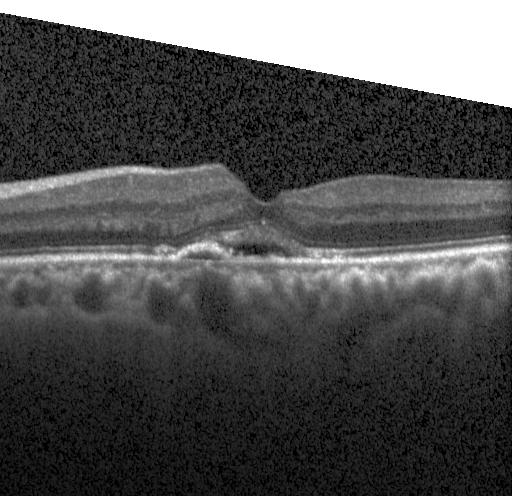
Retinal OCT B-scan; centered on the fovea; SD-OCT; instrument: Heidelberg Spectralis
This B-scan demonstrates CNV.